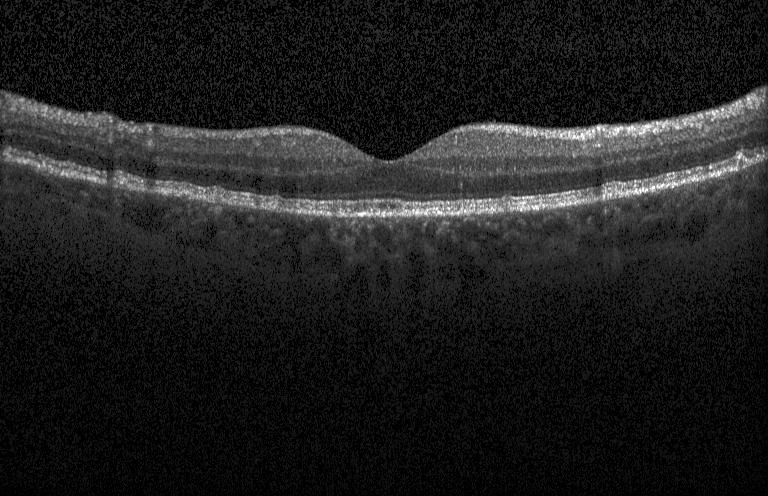

Impression: drusen.